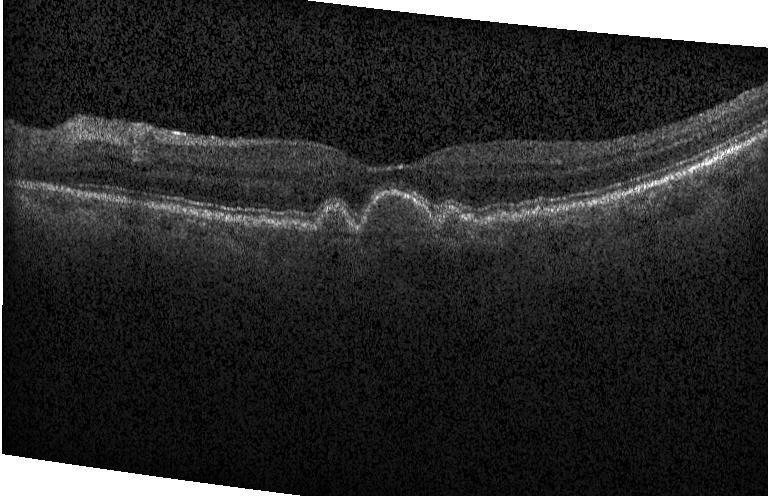

Horizontal scan through the fovea. Retinal OCT B-scan. Drusen.